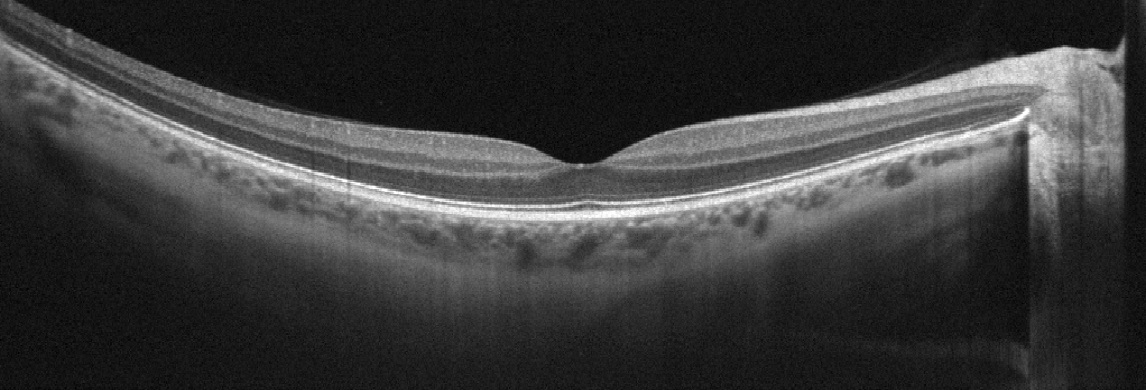
OCT finding: no AMD, DME, ERM, RAO, RVO, or VID.